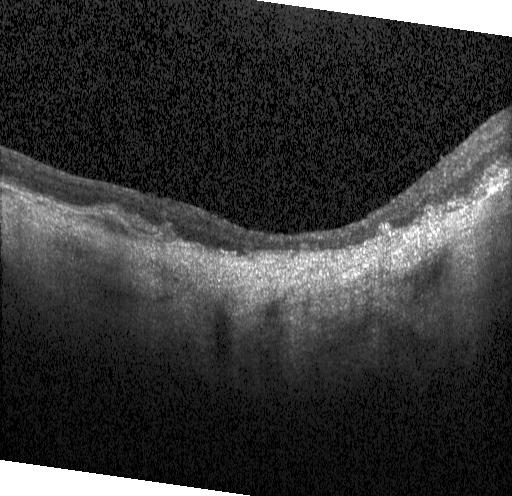 OCT B-scan showing a choroidal neovascular membrane.